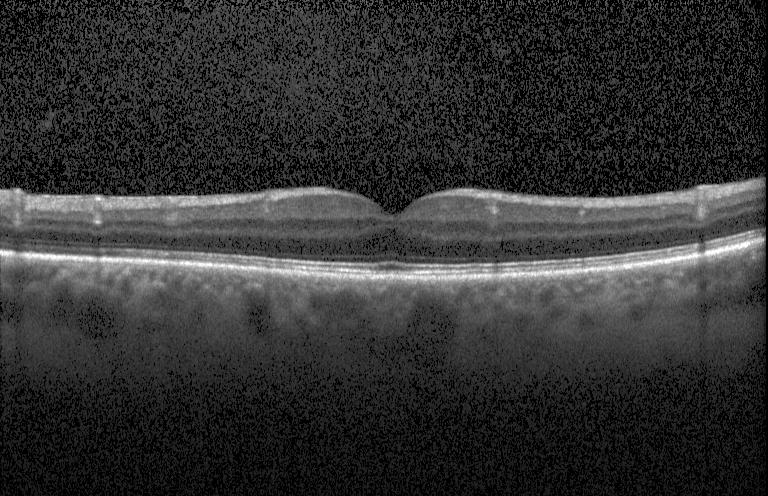
OCT B-scan, macular scan. Finding: no choroidal neovascularization, diabetic macular edema, or drusen.